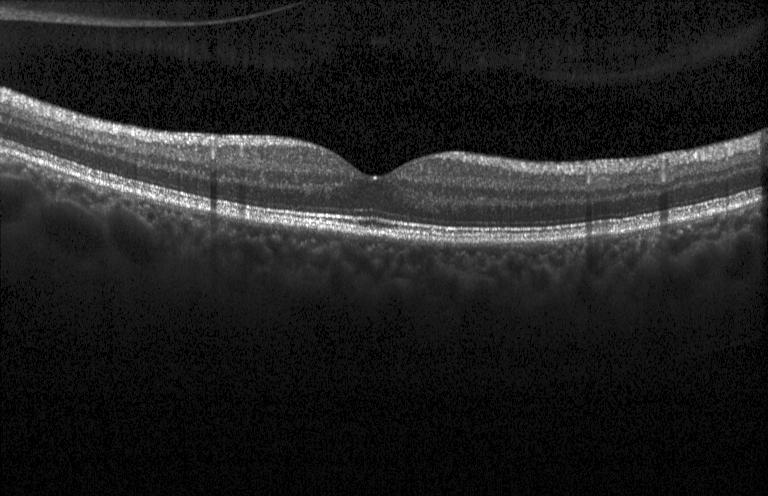 Impression: neither CNV, DME, nor drusen.